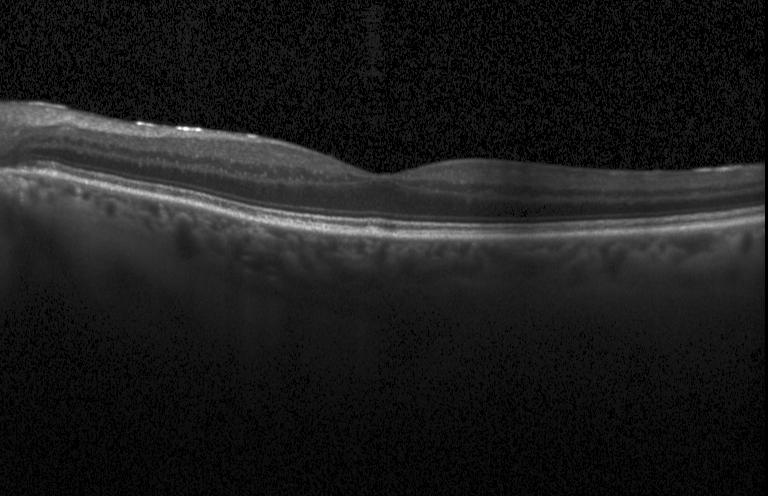
Dx: no evidence of choroidal neovascularization, diabetic macular edema, or drusen.